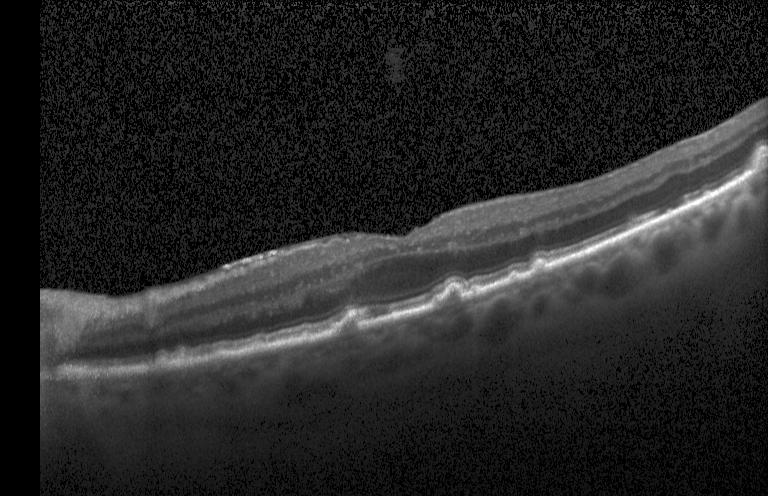
Macular OCT demonstrating sub-RPE drusenoid deposits.